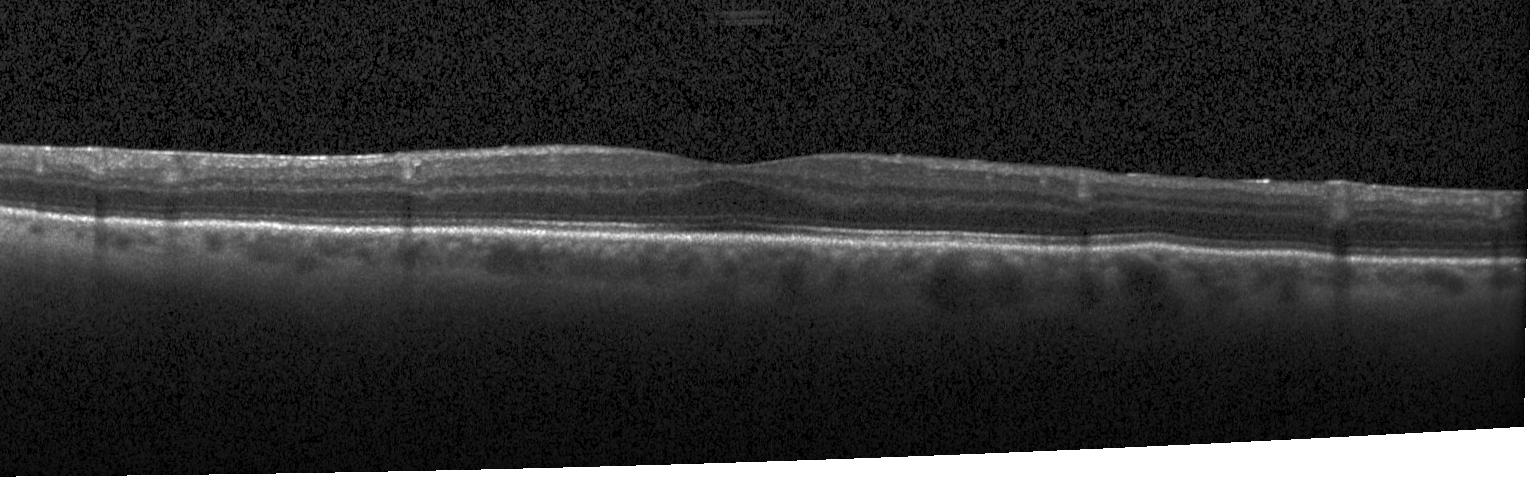 Spectral-domain OCT, macular scan, retinal OCT B-scan — Impression: no choroidal neovascularization, no diabetic macular edema, and no drusen.